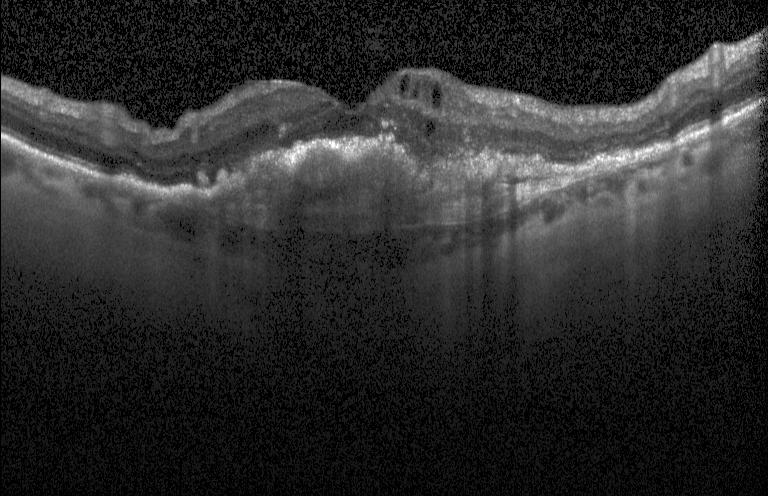
Acquired on a Heidelberg Spectralis. Retinal OCT B-scan
OCT finding: choroidal neovascularization.